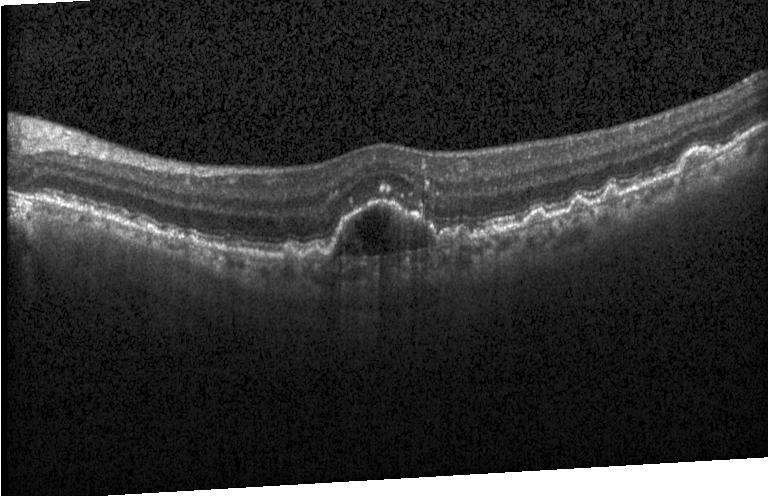

OCT scan showing CNV.